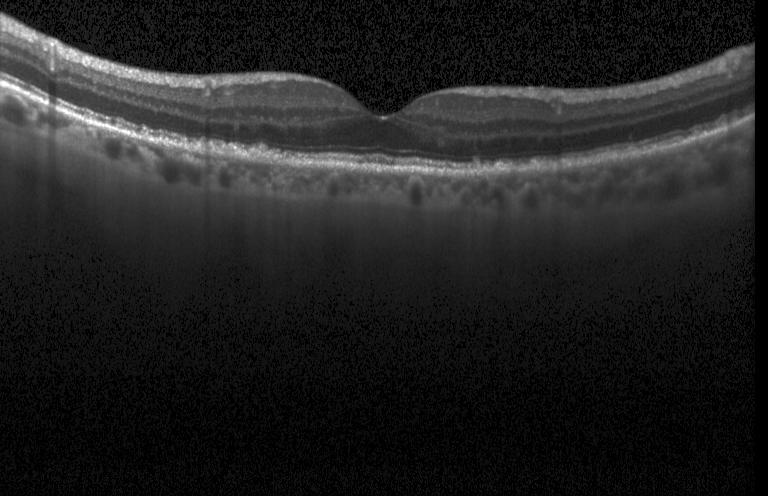

OCT finding: sub-RPE drusenoid deposits.